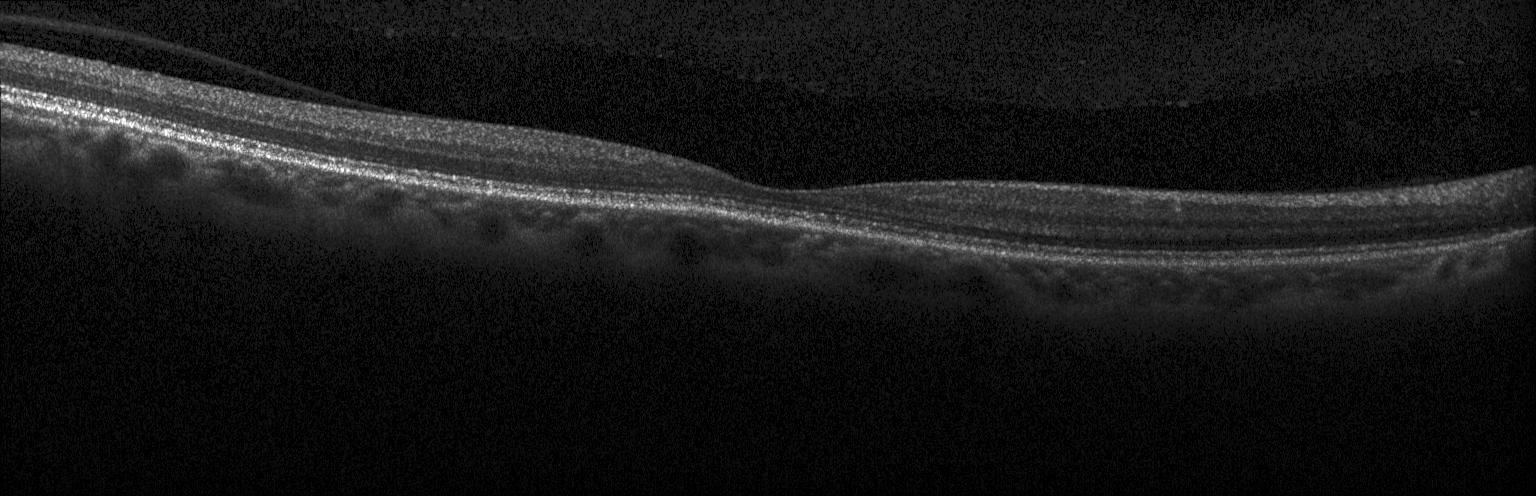
Optical coherence tomography B-scan, instrument: Heidelberg Spectralis, fovea-centered
Finding: no choroidal neovascularization, diabetic macular edema, or drusen.